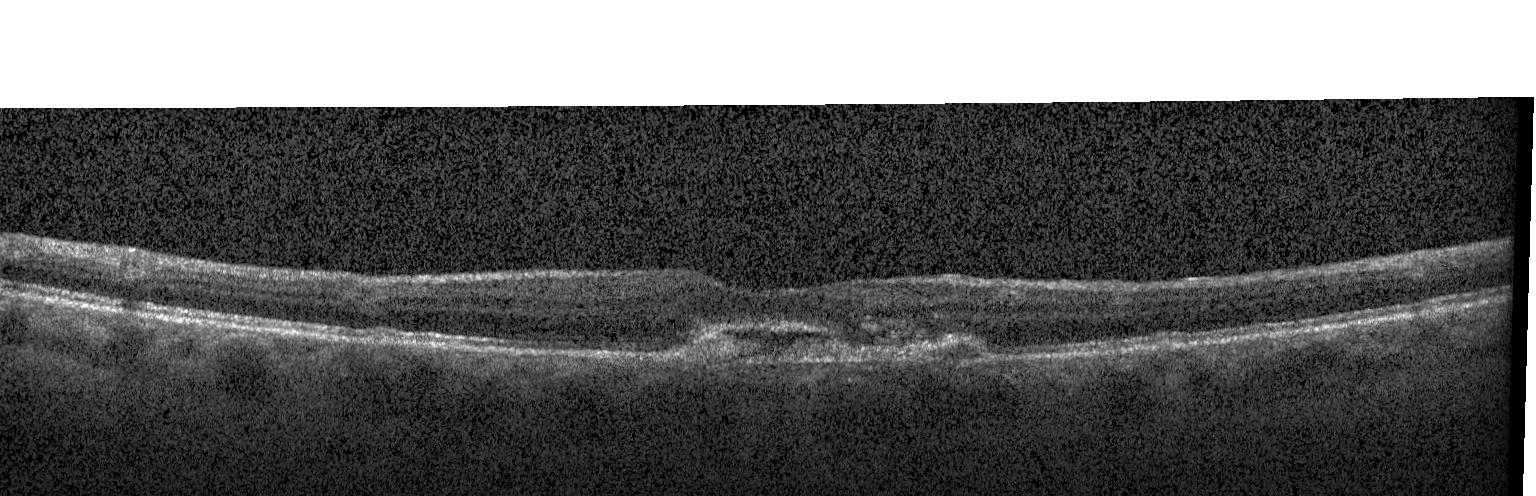 OCT B-scan showing CNV.